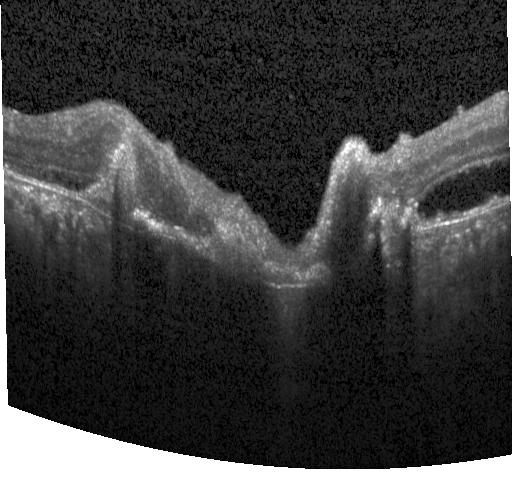 Instrument: Heidelberg Spectralis; horizontal scan through the fovea; OCT line scan; spectral-domain optical coherence tomography. Assessment: choroidal neovascularization.